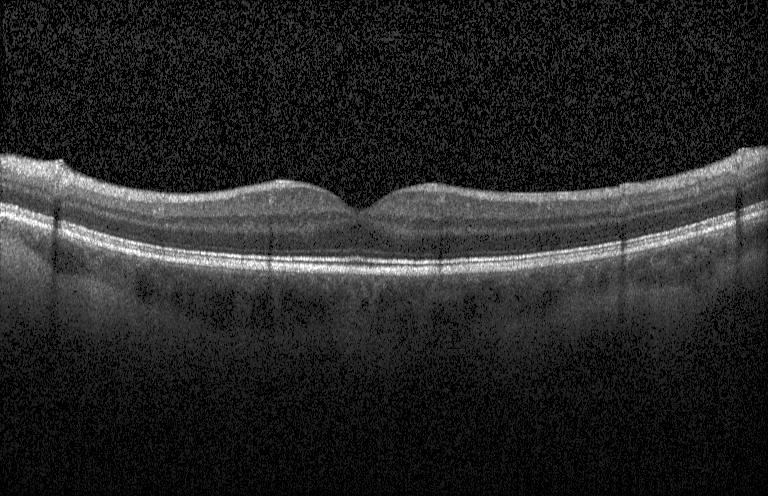
Spectral-domain OCT; fovea-centered; optical coherence tomography scan — Diagnosis: no choroidal neovascularization, no diabetic macular edema, and no drusen.